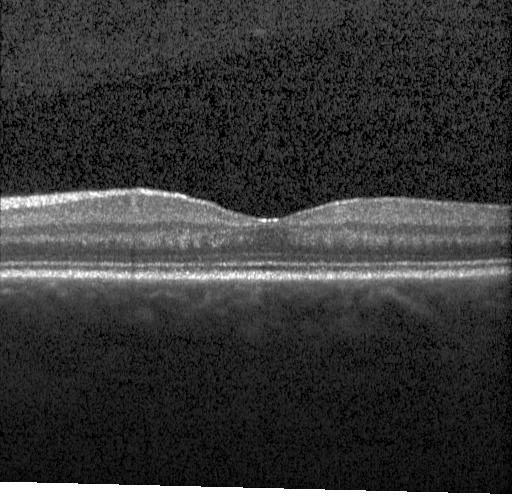 SD-OCT; instrument: Heidelberg Spectralis; OCT line scan
OCT finding: no CNV, no DME, and no drusen.